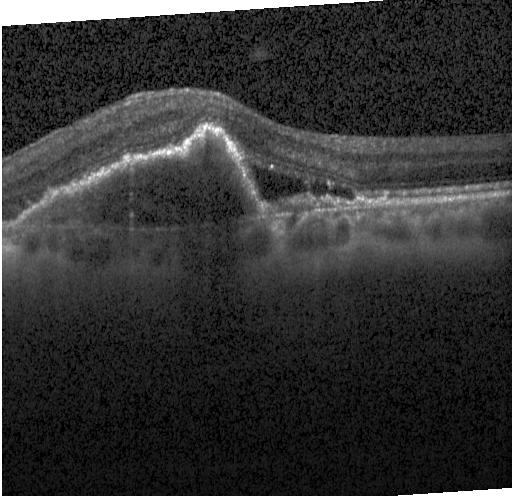

OCT scan showing choroidal neovascularization.